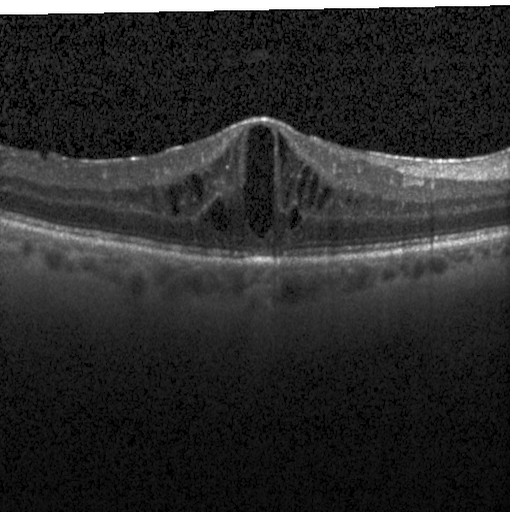
Spectral-domain OCT, fovea-centered, OCT B-scan, Heidelberg Spectralis — Diagnosis: diabetic macular edema.